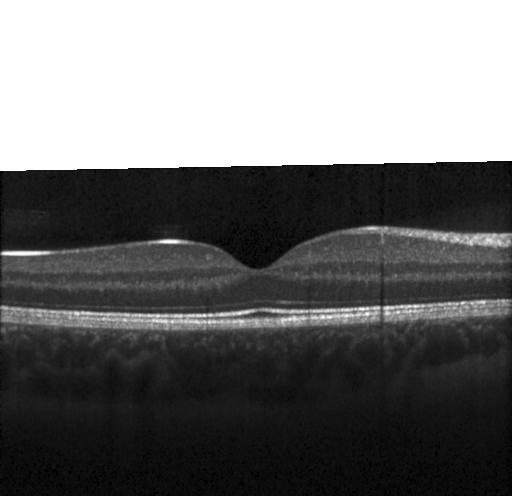
OCT line scan, Heidelberg Spectralis OCT system
Diagnosis: no evidence of choroidal neovascularization, diabetic macular edema, or drusen.